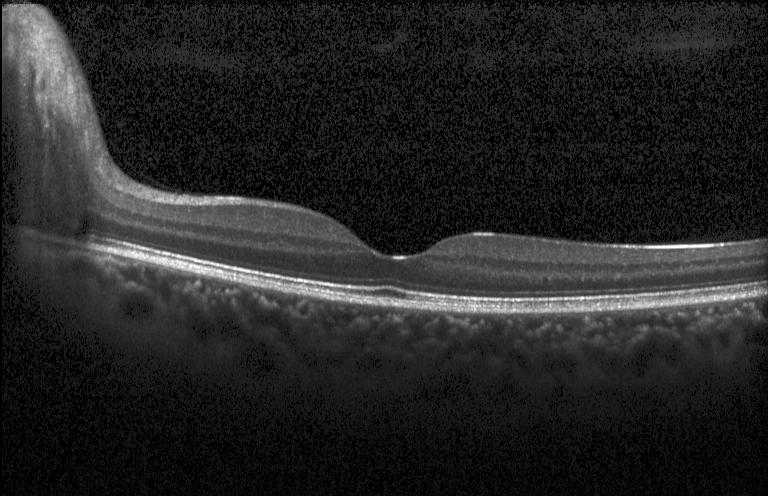

Through the macula, Heidelberg Spectralis, spectral-domain optical coherence tomography, retinal OCT B-scan — The scan shows no choroidal neovascularization, no diabetic macular edema, and no drusen.